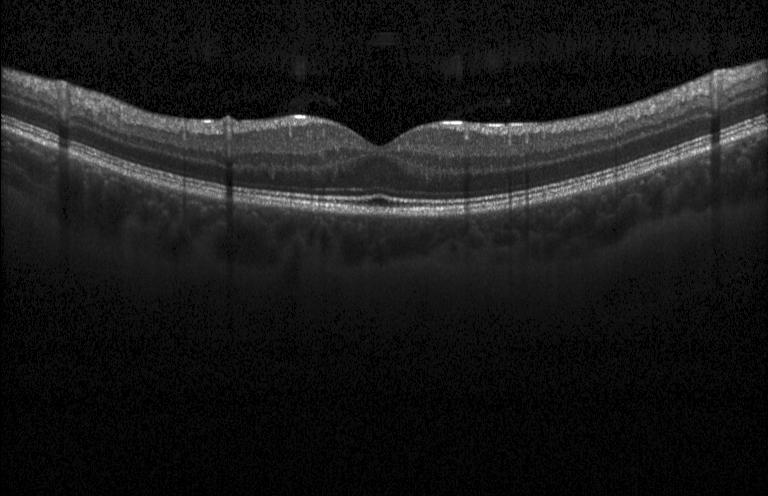 Instrument: Heidelberg Spectralis, retinal OCT cross-section
No evidence of choroidal neovascularization, diabetic macular edema, or drusen.